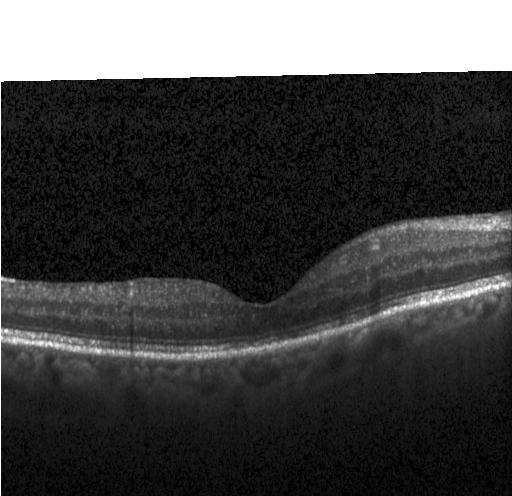 Diagnosis: no choroidal neovascularization, diabetic macular edema, or drusen.